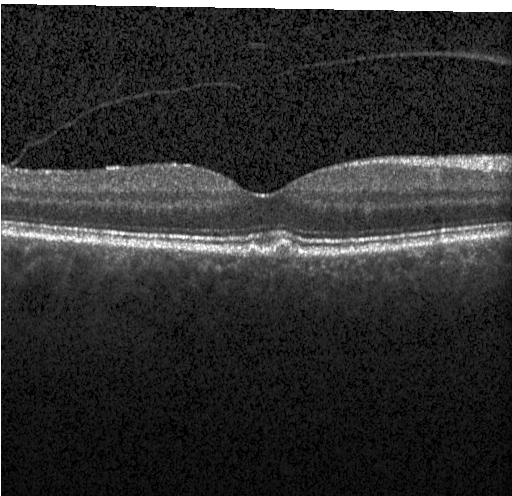

Centered on the fovea; OCT line scan; instrument: Heidelberg Spectralis — Dx: multiple drusen.